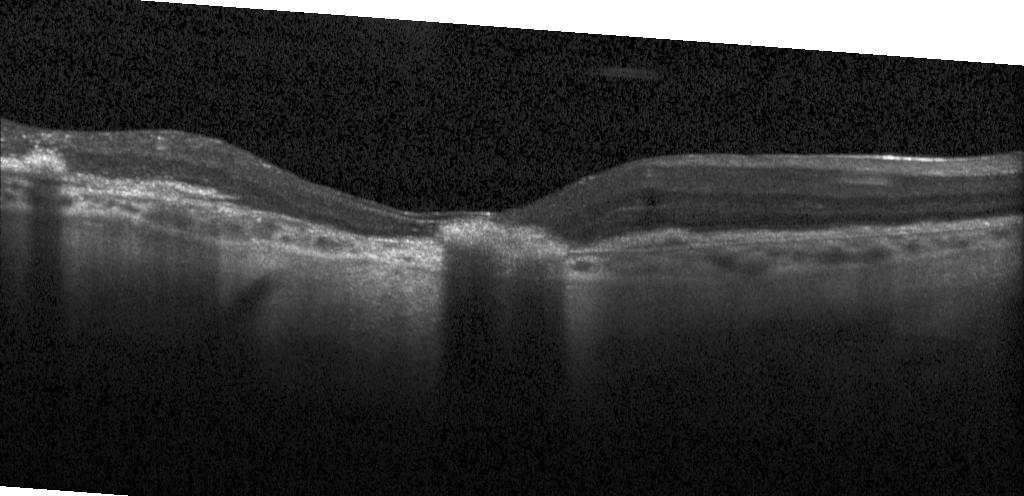 Optical coherence tomography scan
Assessment: CNV.